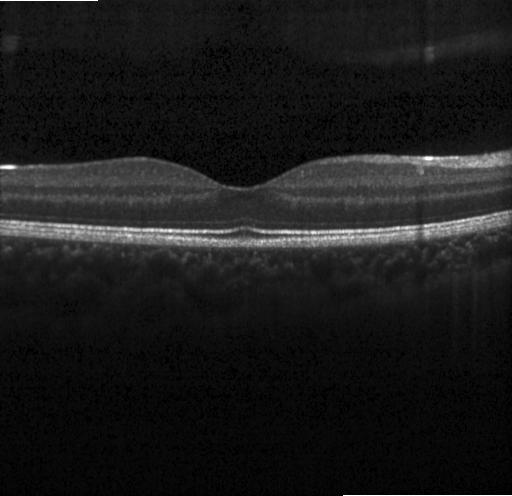 The scan shows no evidence of CNV, DME, or drusen.